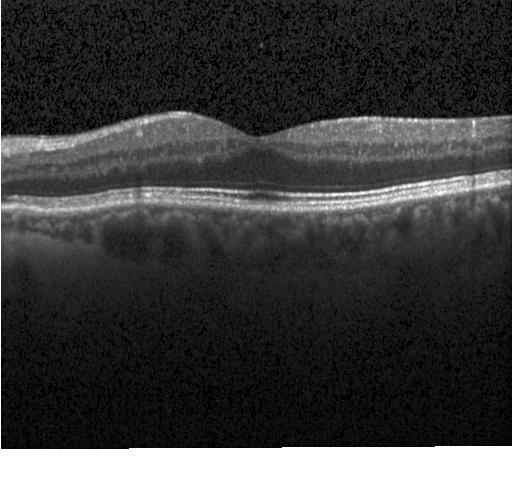 Retinal OCT B-scan · horizontal scan through the fovea
Diagnosis: no evidence of choroidal neovascularization, diabetic macular edema, or drusen.